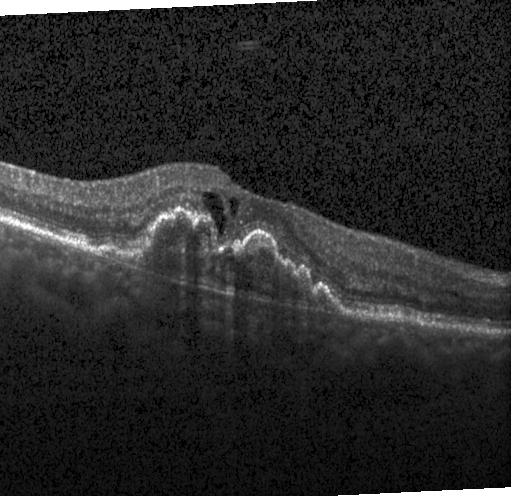
Optical coherence tomography B-scan · SD-OCT · instrument: Heidelberg Spectralis
Impression: choroidal neovascularization (CNV).